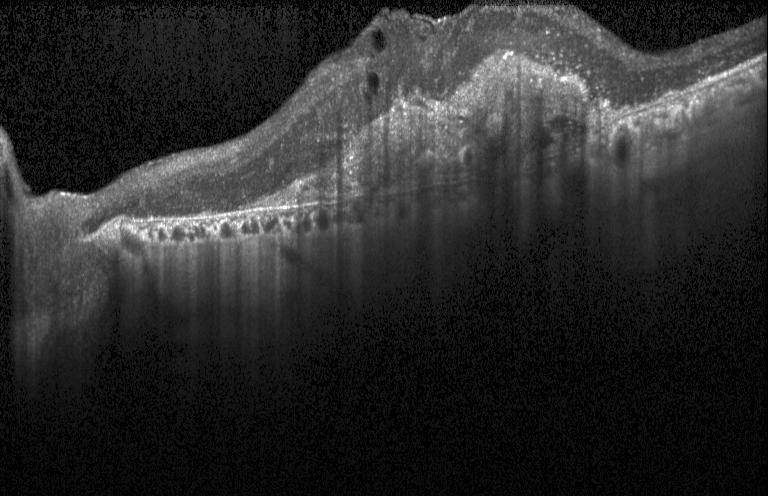
OCT B-scan
Impression: a choroidal neovascular membrane.